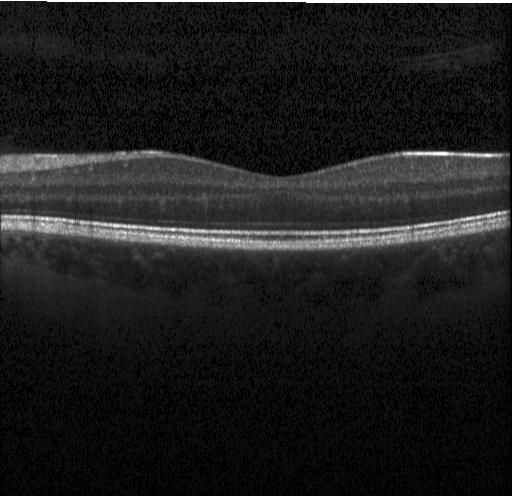 OCT finding: no choroidal neovascularization, no diabetic macular edema, and no drusen.